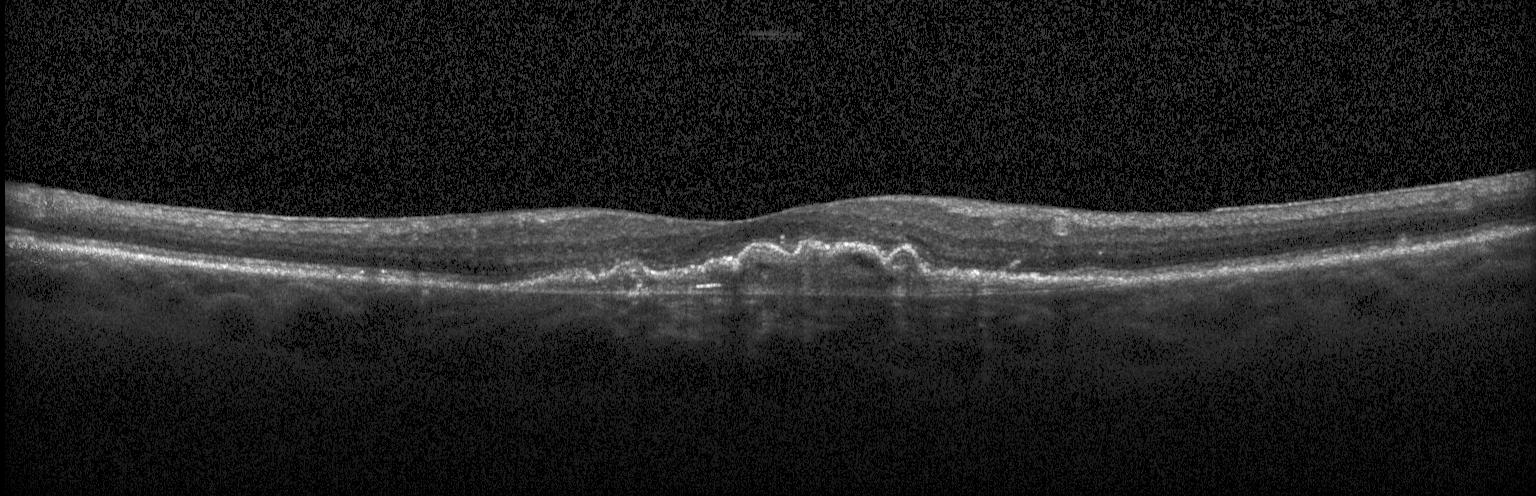

Optical coherence tomography scan; centered on the fovea; SD-OCT — Diagnosis: a choroidal neovascular membrane.